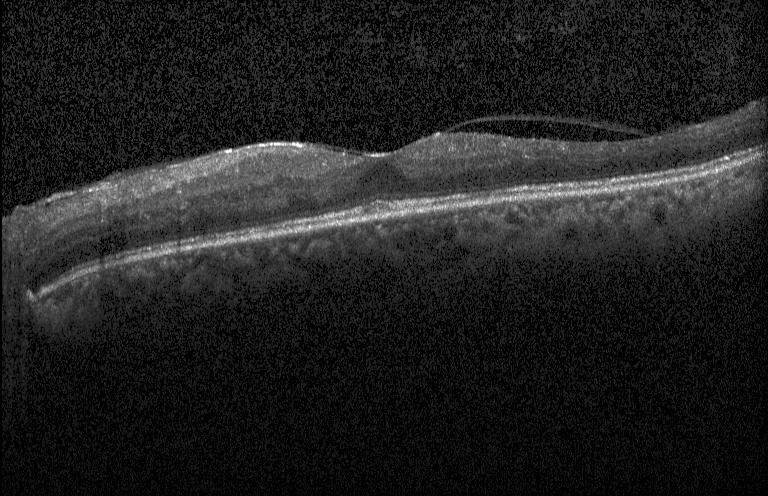
Retinal OCT cross-section.
Impression: DME.